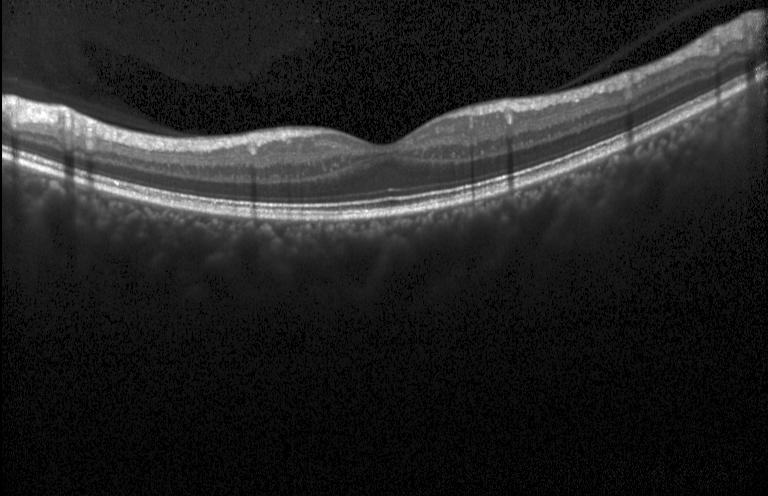

Centered on the fovea. Spectral-domain optical coherence tomography. Retinal OCT cross-section — Impression: no CNV, DME, or drusen.